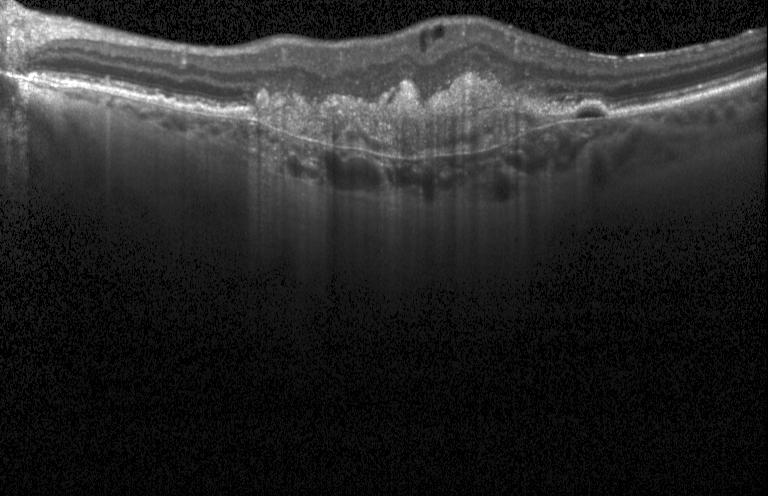 OCT B-scan · acquired on a Heidelberg Spectralis · spectral-domain OCT · macular scan.
The scan shows choroidal neovascularization (CNV).